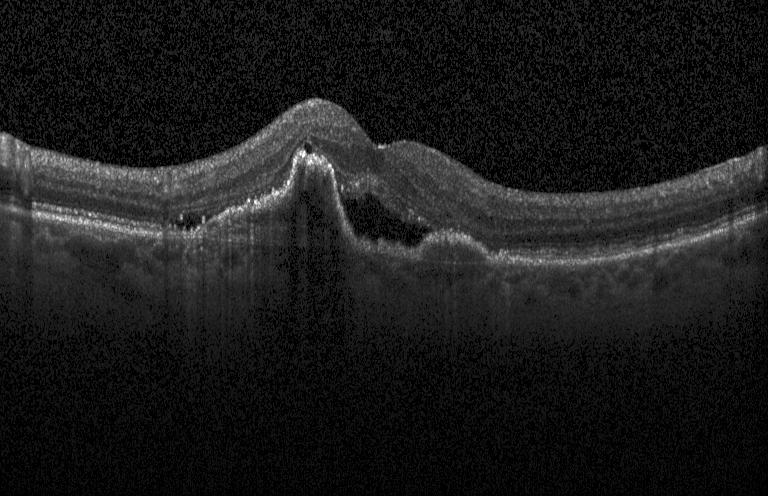

Centered on the fovea, instrument: Heidelberg Spectralis, retinal OCT cross-section — Diagnosis: a choroidal neovascular membrane.